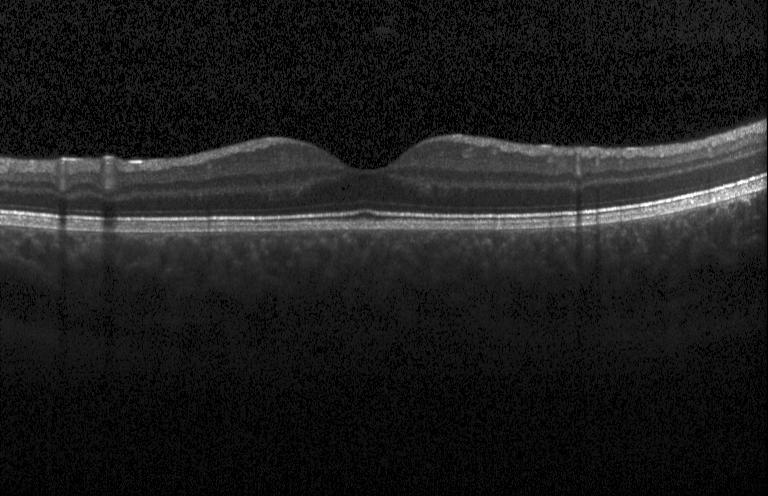 OCT line scan — Dx: no CNV, DME, or drusen.